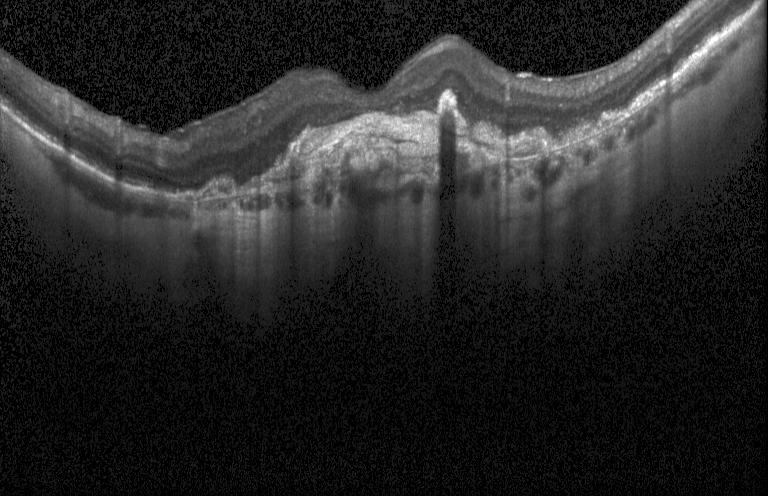
Fovea-centered. Optical coherence tomography scan — OCT finding: a choroidal neovascular membrane.